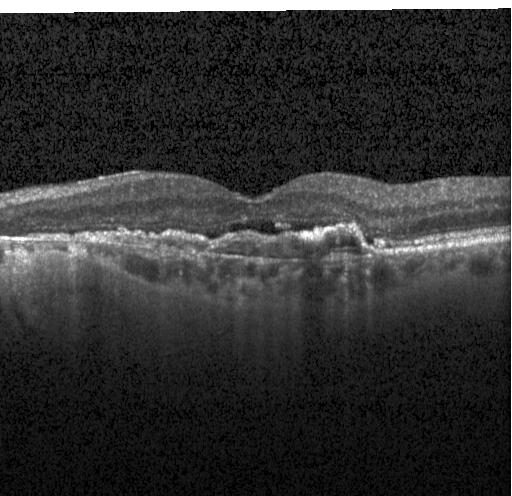

OCT finding: choroidal neovascularization.